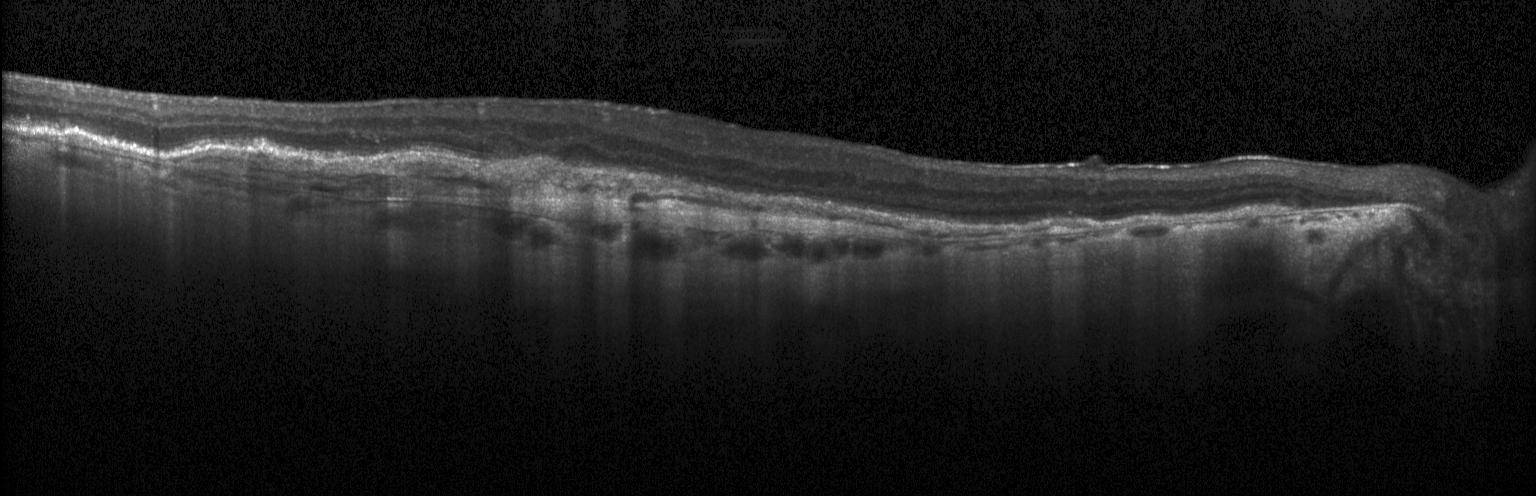 Impression: choroidal neovascularization (CNV).